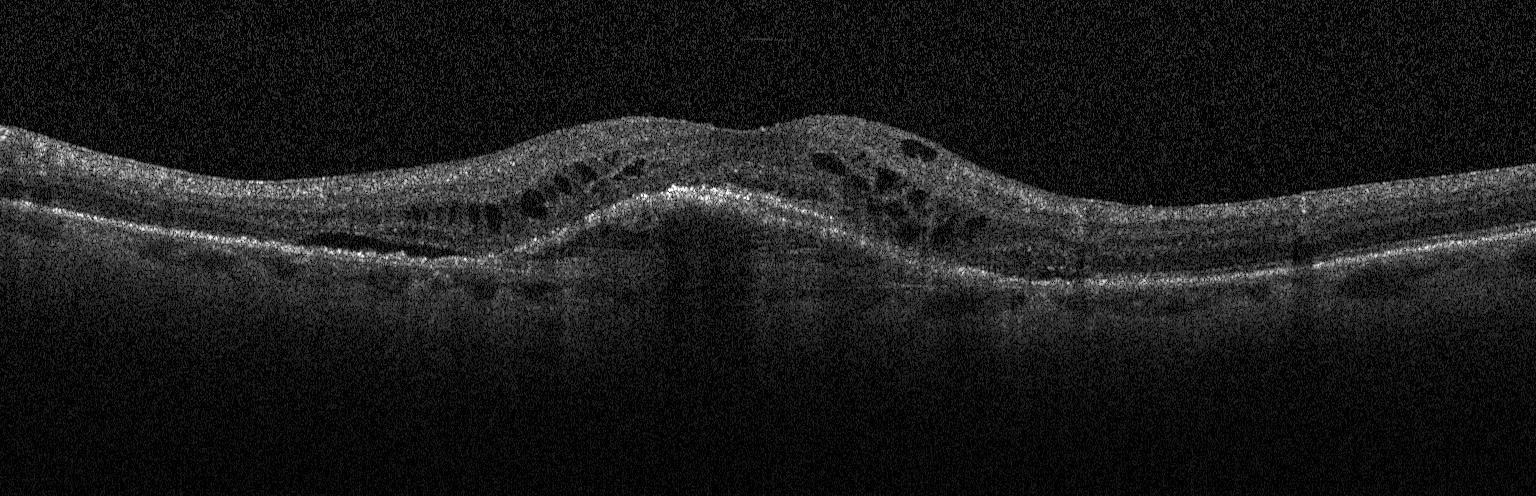 Heidelberg Spectralis OCT system. Spectral-domain OCT. Optical coherence tomography B-scan. Fovea-centered
The scan shows a choroidal neovascular membrane.